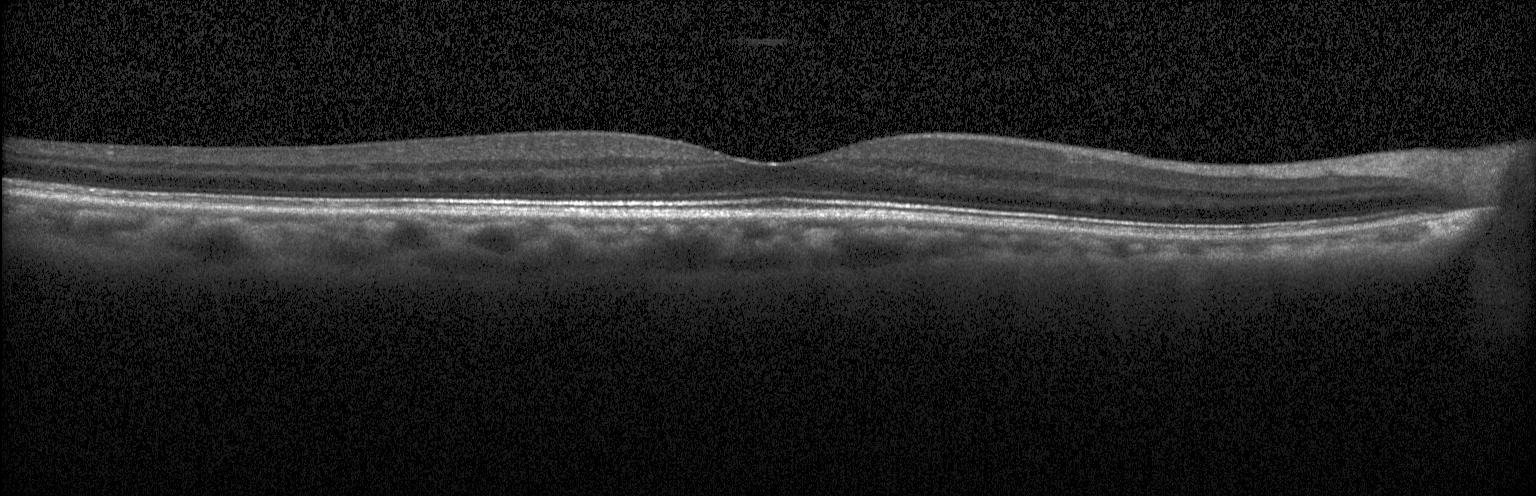 OCT B-scan showing no choroidal neovascularization, diabetic macular edema, or drusen.